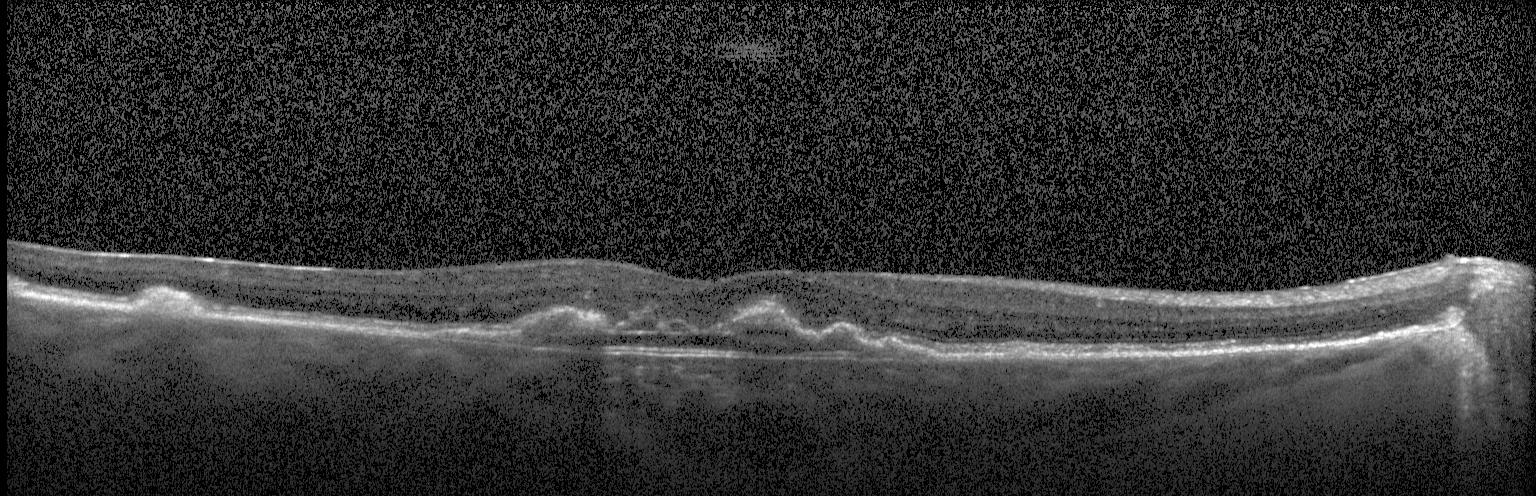 Dx: choroidal neovascularization (CNV).